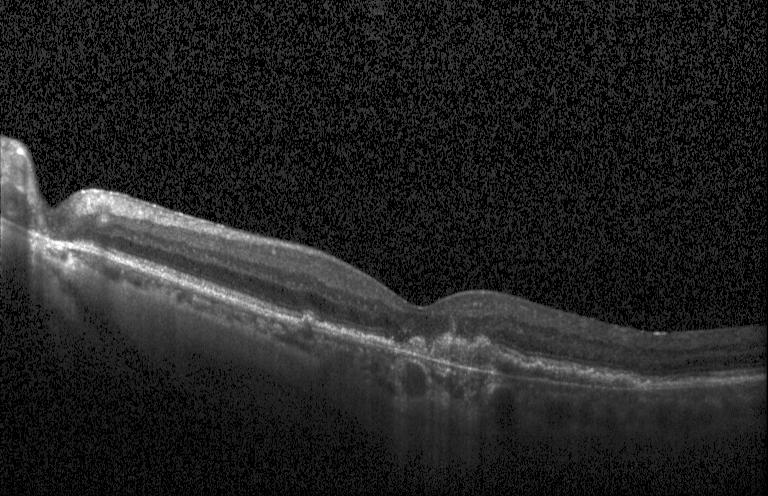
This B-scan demonstrates choroidal neovascularization (CNV).